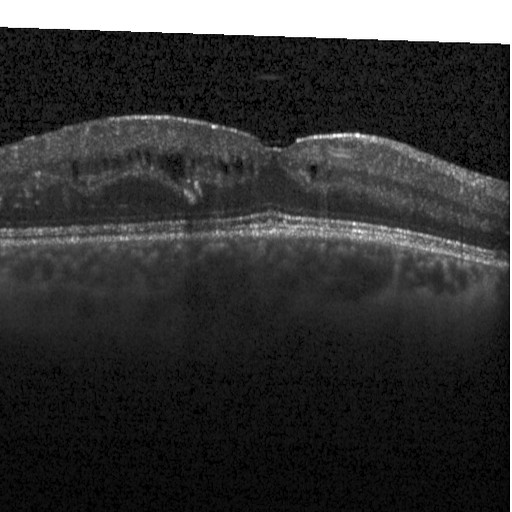
Retinal OCT cross-section. Macular scan. Spectral-domain OCT. DME.